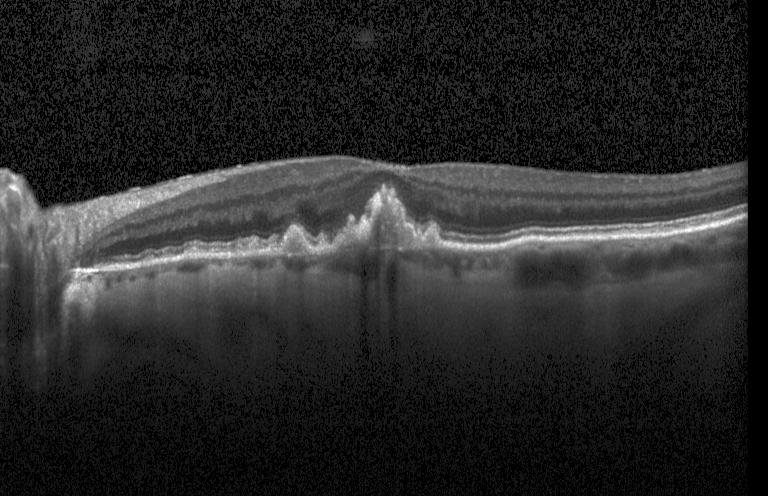 Retinal OCT B-scan.
Finding: choroidal neovascularization (CNV).